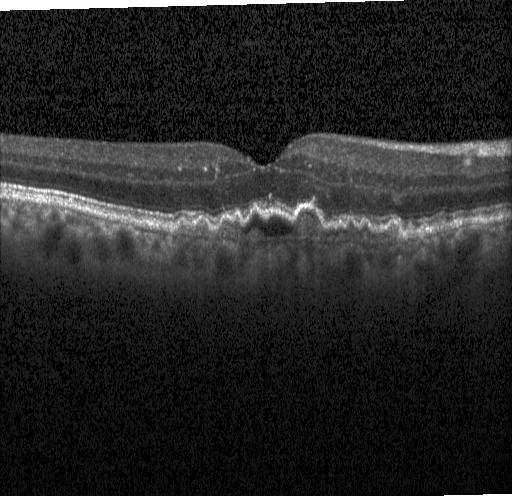

Optical coherence tomography scan, Heidelberg Spectralis OCT system. Finding: a choroidal neovascular membrane.